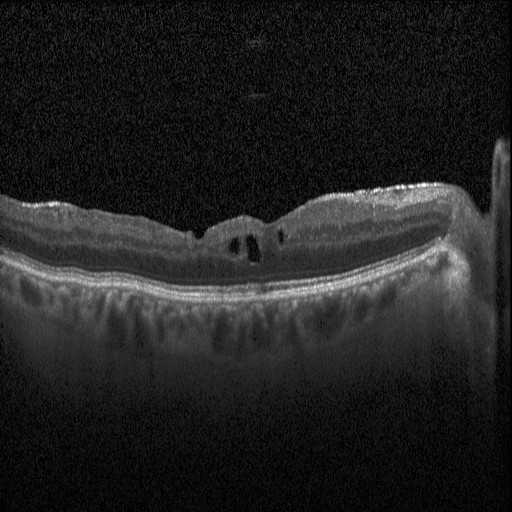

Retinal OCT cross-section · Heidelberg Spectralis OCT system.
Macular OCT: DME.